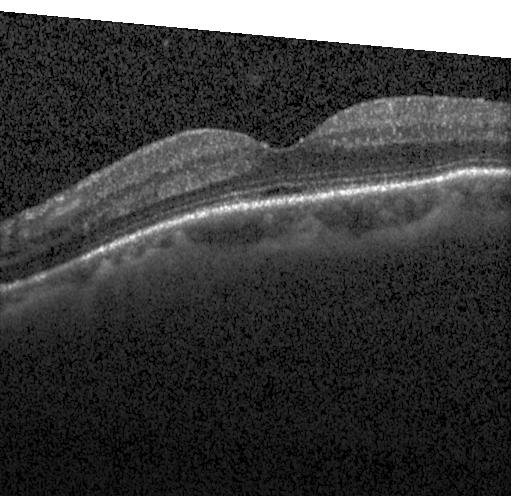

Centered on the fovea; OCT line scan. Diagnosis: no evidence of choroidal neovascularization, diabetic macular edema, or drusen.